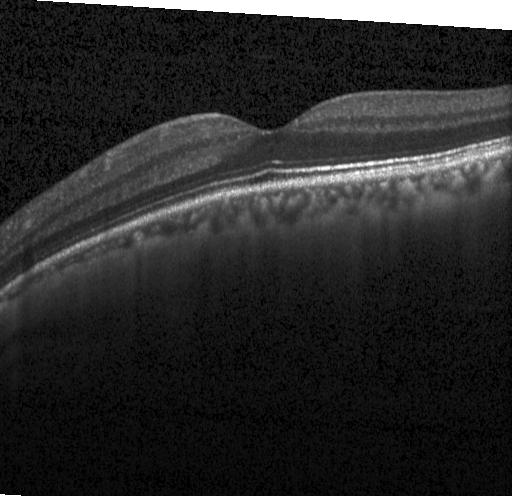

Retinal OCT cross-section · spectral-domain optical coherence tomography. OCT finding: neither CNV, DME, nor drusen.